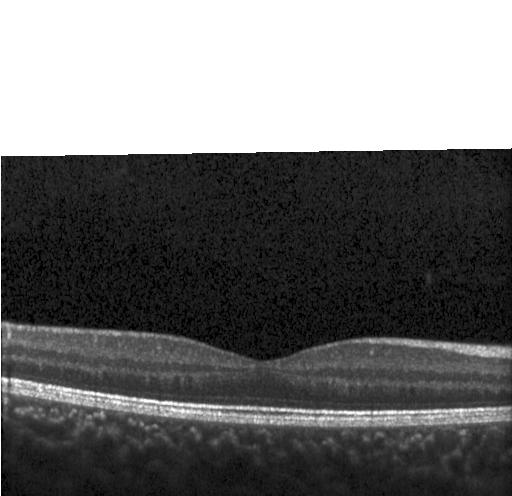
Through the macula, instrument: Heidelberg Spectralis, retinal OCT B-scan. This B-scan demonstrates no evidence of CNV, DME, or drusen.